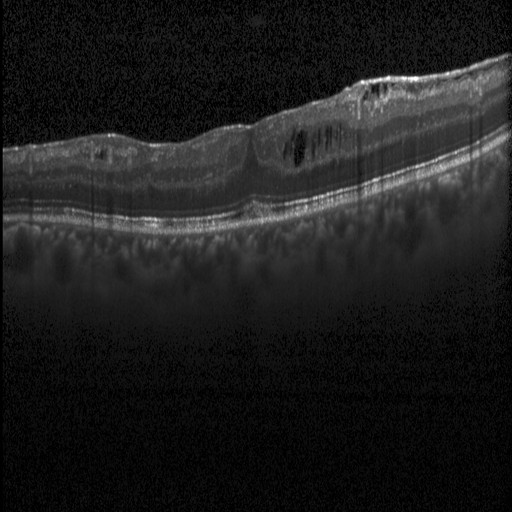

Optical coherence tomography B-scan, macular scan.
Diabetic macular edema.